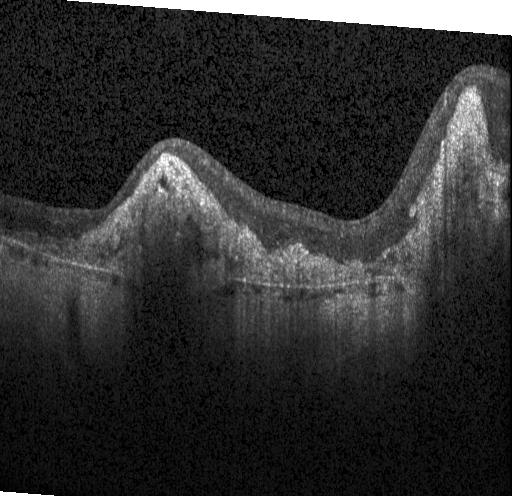 Finding: a choroidal neovascular membrane.